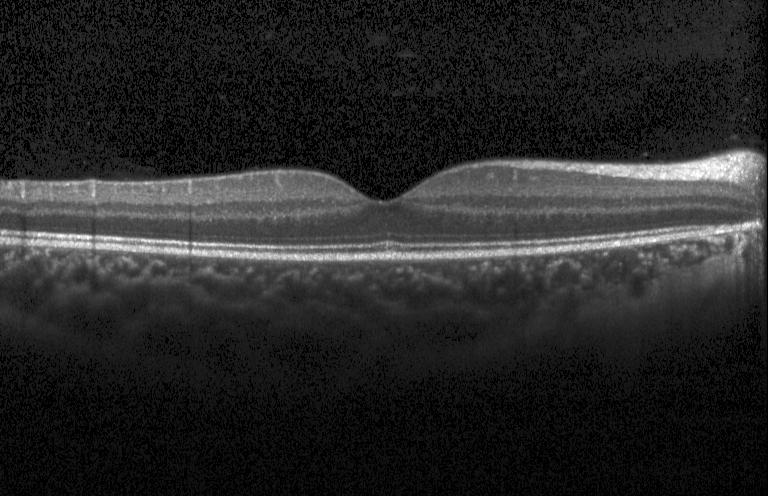 SD-OCT; retinal OCT cross-section — Impression: neither choroidal neovascularization, diabetic macular edema, nor drusen.